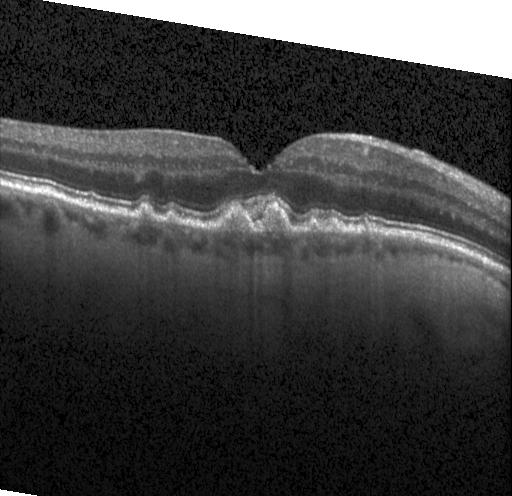

OCT B-scan, macular scan, spectral-domain optical coherence tomography. Drusen.